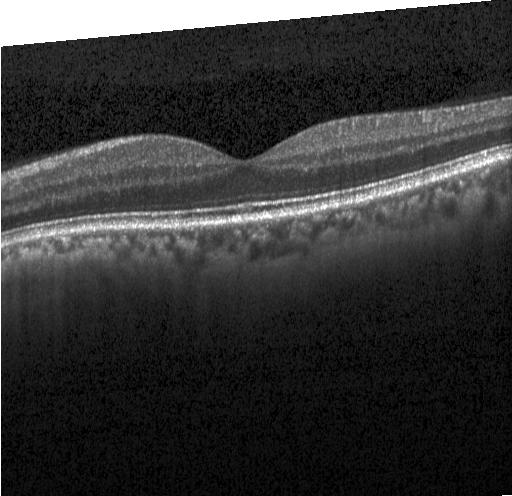
Finding: neither choroidal neovascularization, diabetic macular edema, nor drusen.